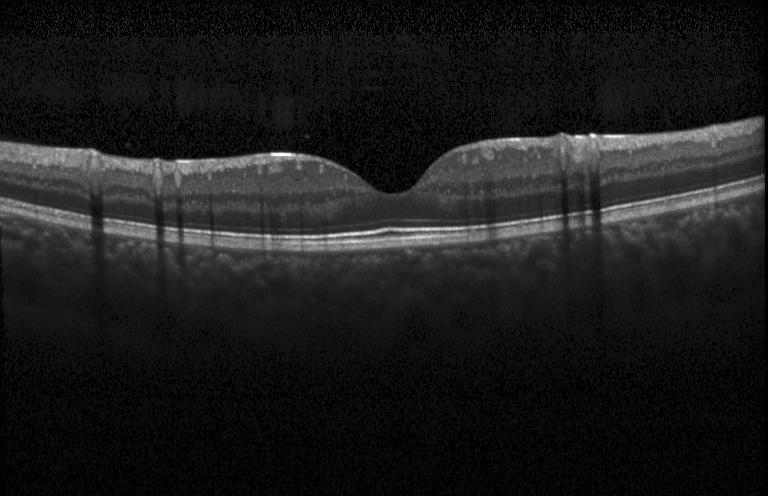 Diagnosis: neither choroidal neovascularization, diabetic macular edema, nor drusen.